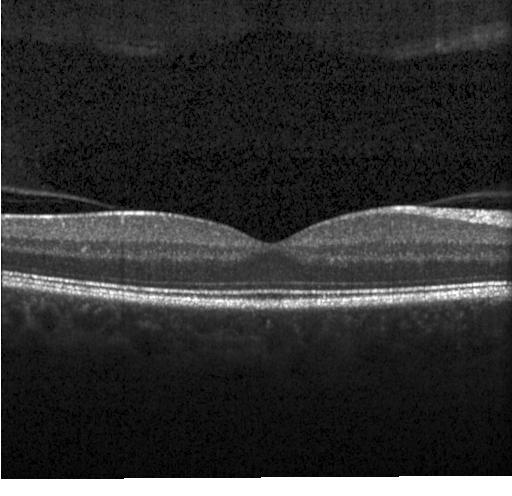

Spectral-domain OCT B-scan: neither choroidal neovascularization, diabetic macular edema, nor drusen.